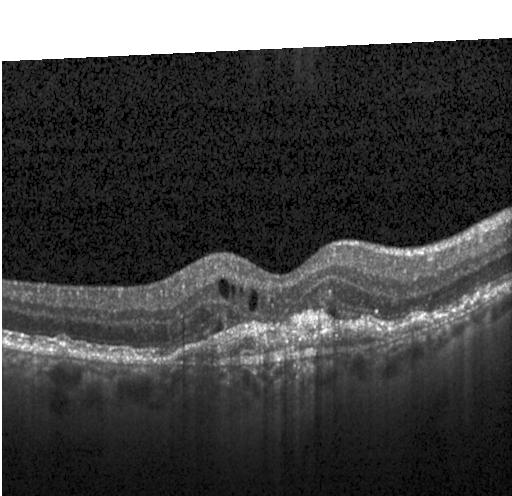
OCT line scan — Impression: a choroidal neovascular membrane.